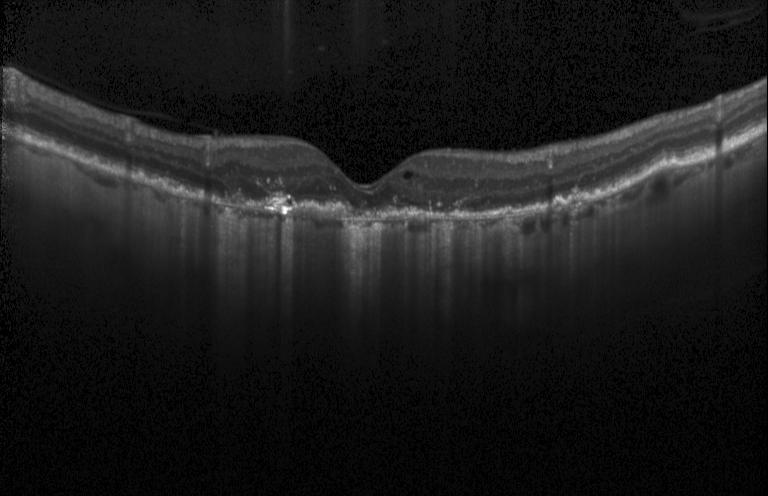

OCT B-scan; spectral-domain optical coherence tomography; centered on the fovea; Heidelberg Spectralis. A choroidal neovascular membrane.